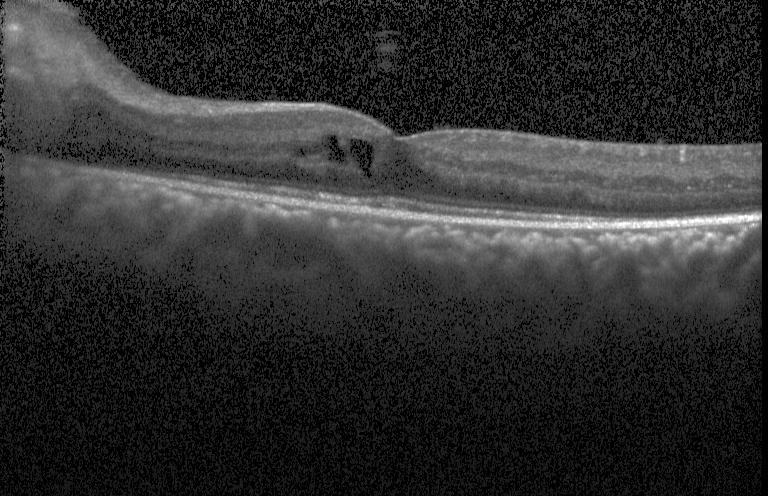 Spectral-domain OCT · instrument: Heidelberg Spectralis · OCT line scan
Diabetic macular edema (DME).